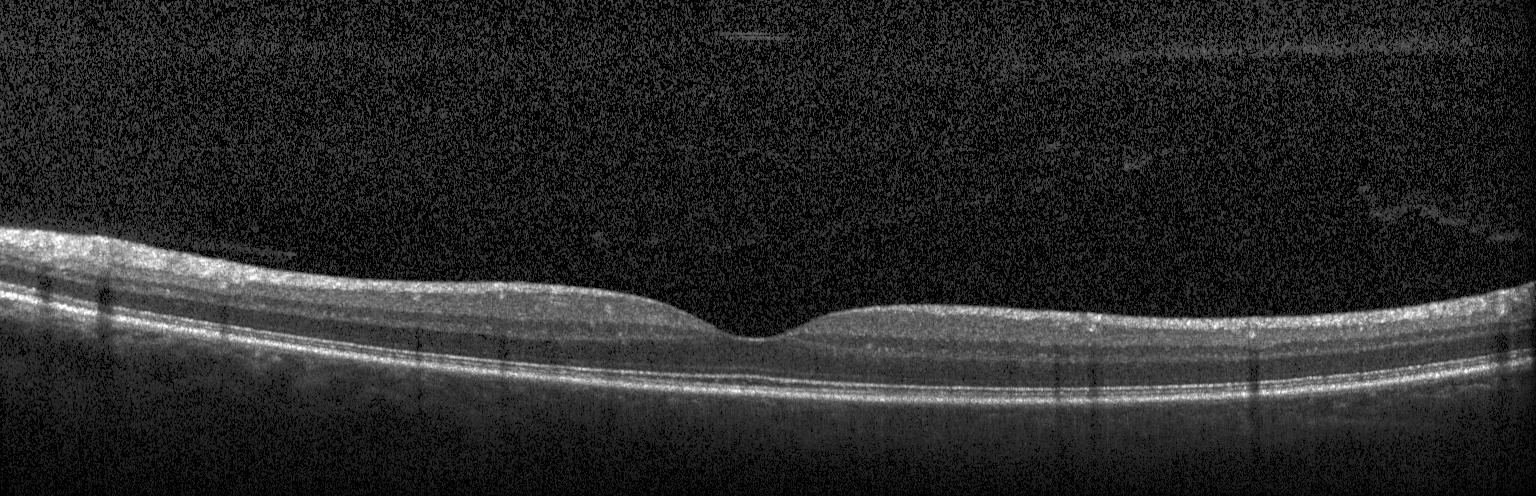
Instrument: Heidelberg Spectralis. Spectral-domain OCT. Retinal OCT cross-section — Impression: neither CNV, DME, nor drusen.